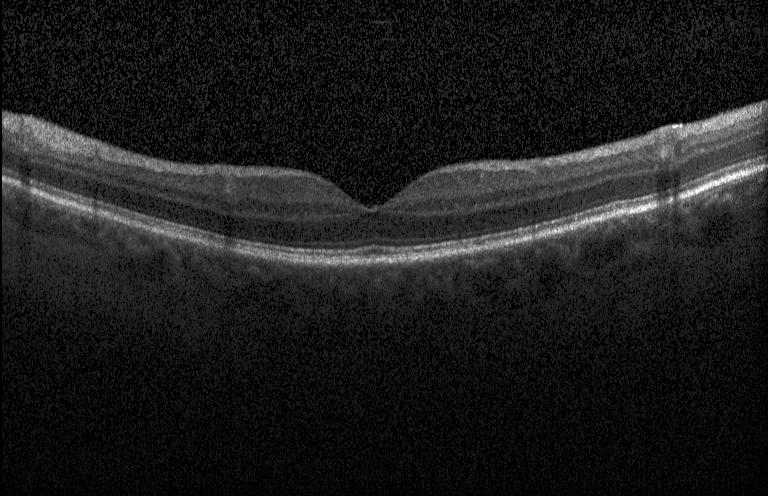
Horizontal scan through the fovea; SD-OCT; retinal OCT B-scan; acquired on a Heidelberg Spectralis.
Macular OCT: no choroidal neovascularization, diabetic macular edema, or drusen.